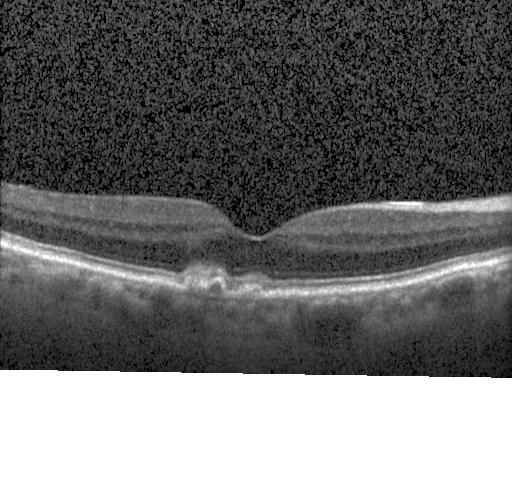
Multiple drusen.